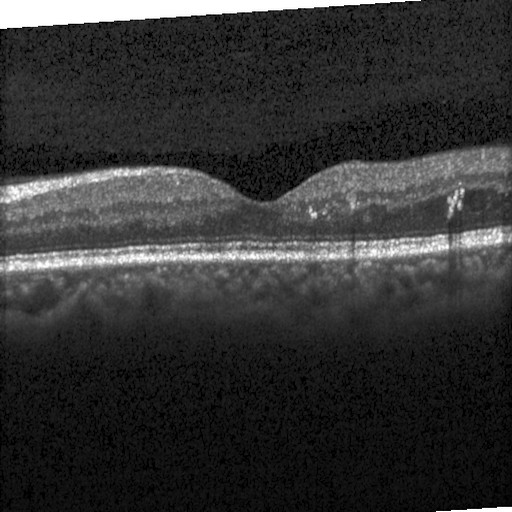

Heidelberg Spectralis. Retinal OCT B-scan. Horizontal scan through the fovea. Spectral-domain optical coherence tomography.
Finding: diabetic macular edema.